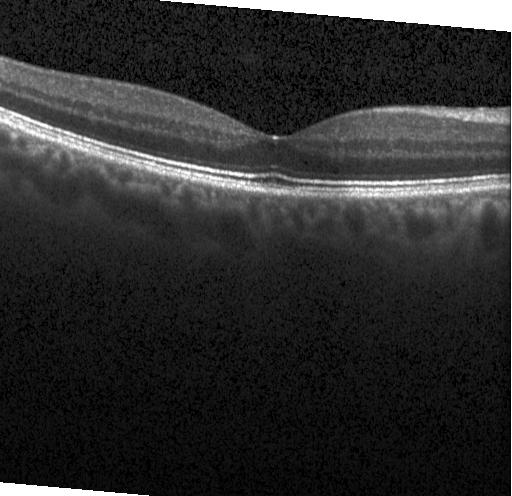
Optical coherence tomography B-scan
This B-scan demonstrates no evidence of choroidal neovascularization, diabetic macular edema, or drusen.